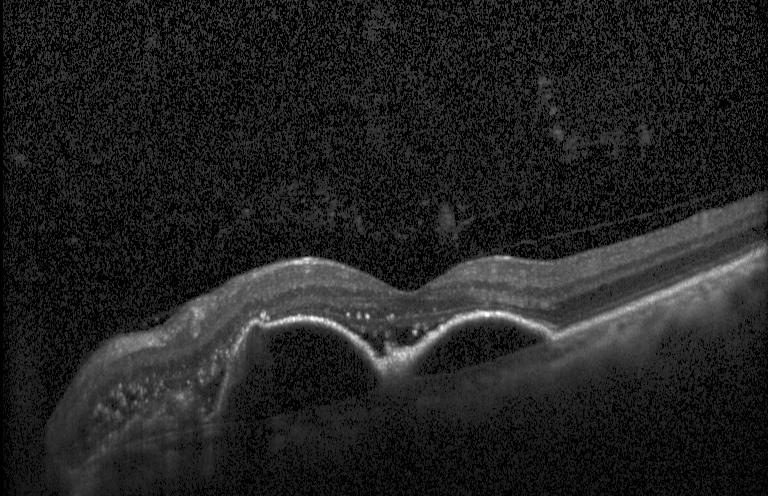

Spectral-domain OCT B-scan: a choroidal neovascular membrane.